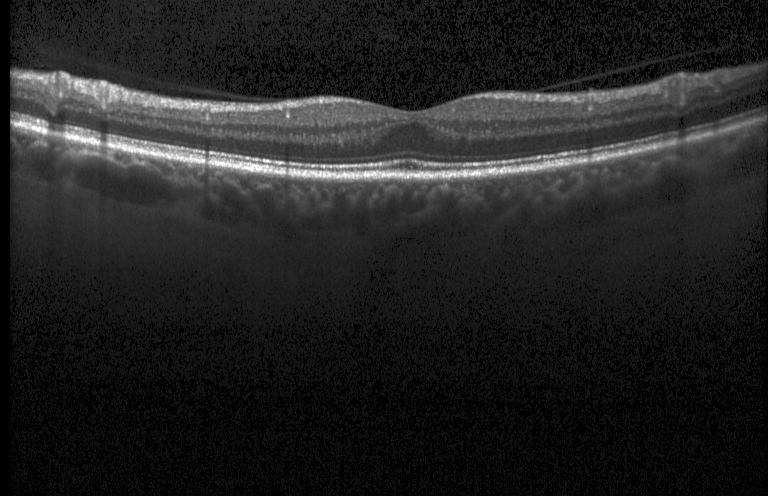
This B-scan demonstrates neither choroidal neovascularization, diabetic macular edema, nor drusen.